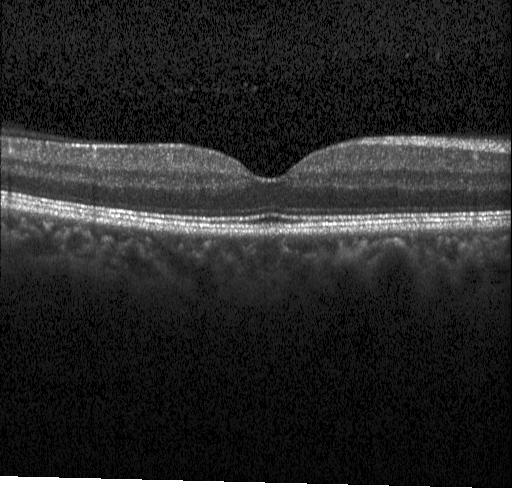 The scan shows no CNV, DME, or drusen.